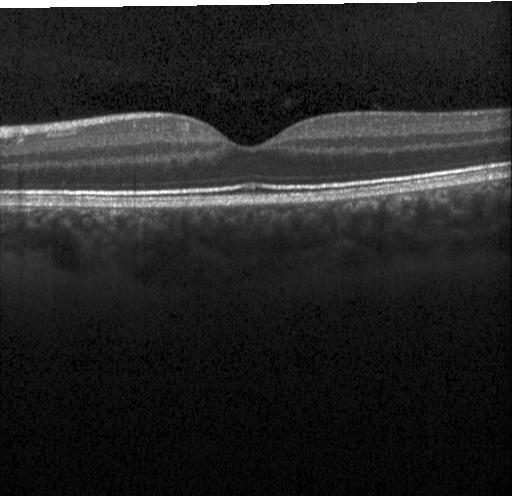

OCT B-scan. SD-OCT
Impression: neither choroidal neovascularization, diabetic macular edema, nor drusen.